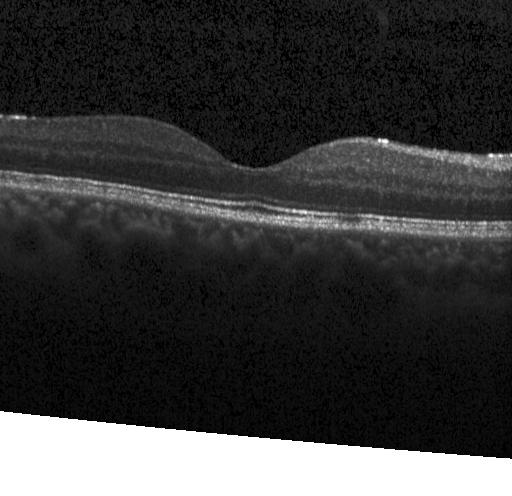 Heidelberg Spectralis. Retinal OCT B-scan
This B-scan demonstrates no CNV, DME, or drusen.